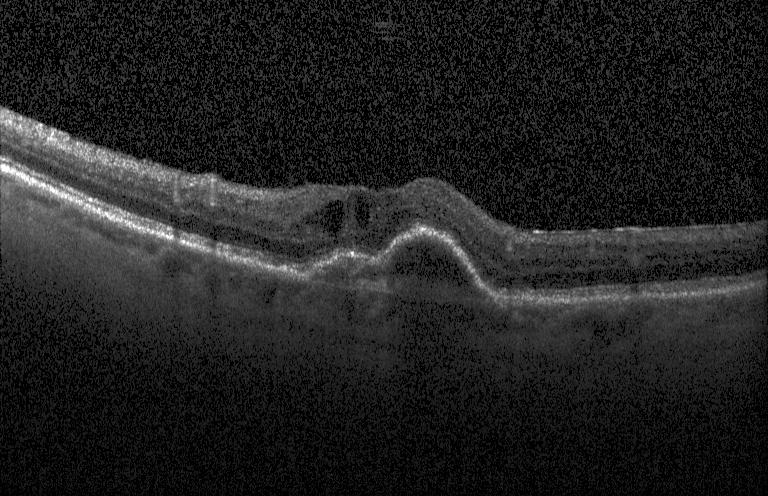 OCT line scan
Diagnosis: choroidal neovascularization (CNV).